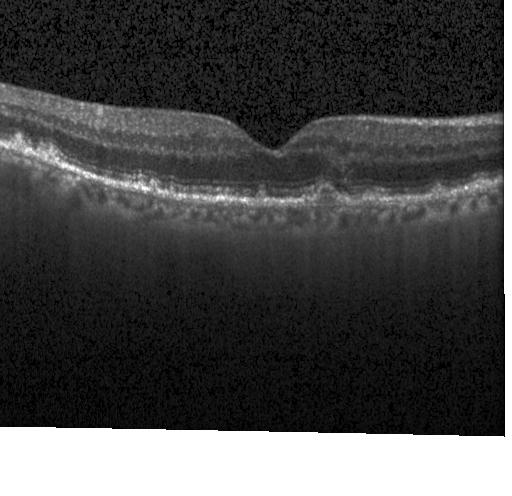 OCT finding: sub-RPE drusenoid deposits.